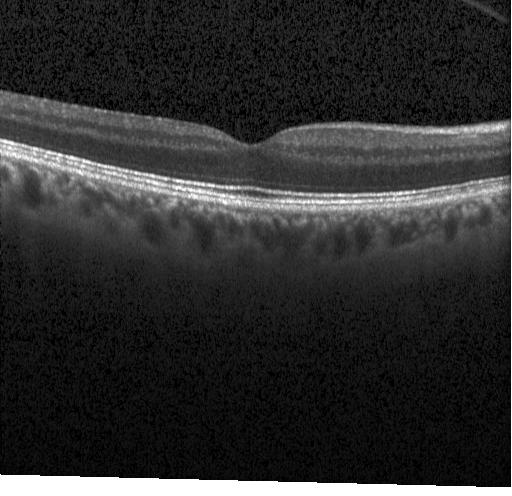
Diagnosis: no evidence of choroidal neovascularization, diabetic macular edema, or drusen.